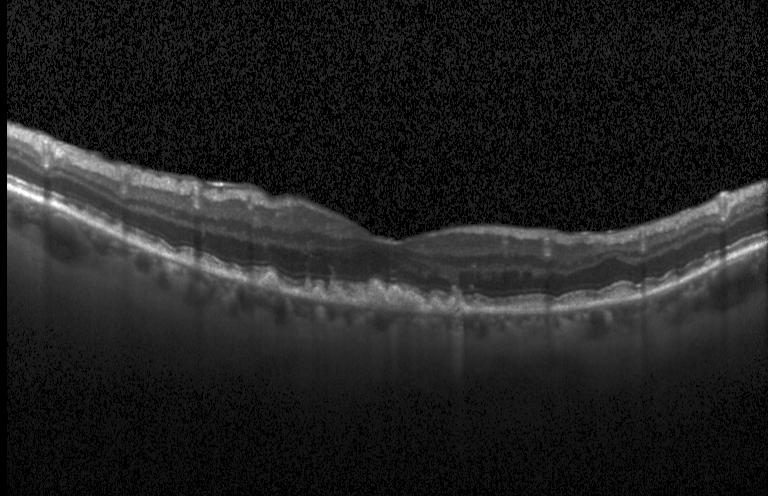 Optical coherence tomography scan · spectral-domain optical coherence tomography · instrument: Heidelberg Spectralis · horizontal scan through the fovea.
Drusen.